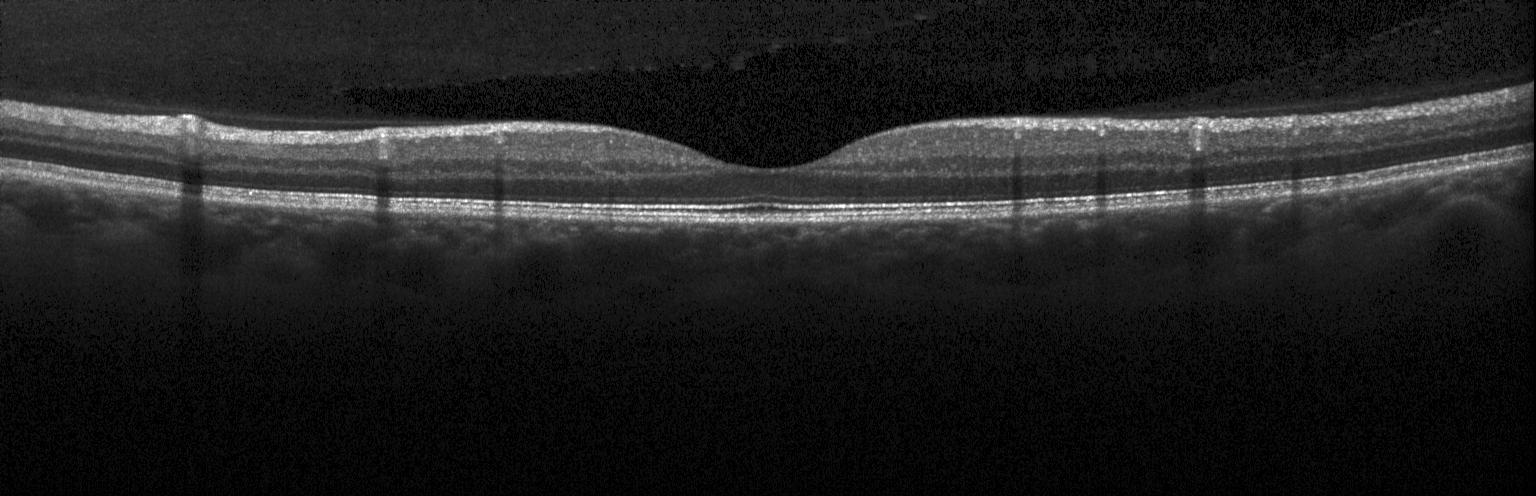
Heidelberg Spectralis · retinal OCT cross-section · SD-OCT · fovea-centered
Finding: no evidence of choroidal neovascularization, diabetic macular edema, or drusen.